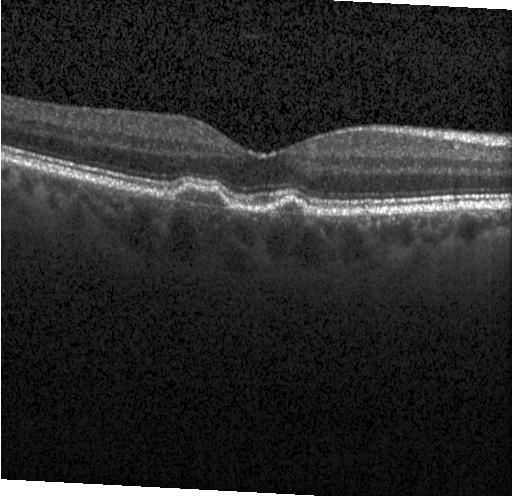

Retinal OCT cross-section.
Diagnosis: multiple drusen.